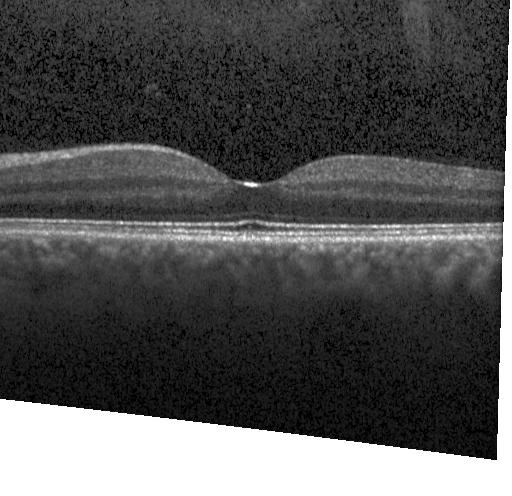

Optical coherence tomography scan
Diagnosis: no CNV, no DME, and no drusen.